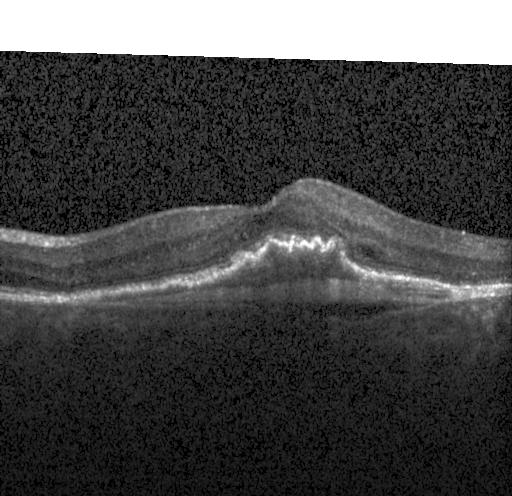
Optical coherence tomography B-scan, fovea-centered, Heidelberg Spectralis.
Diagnosis: a choroidal neovascular membrane.